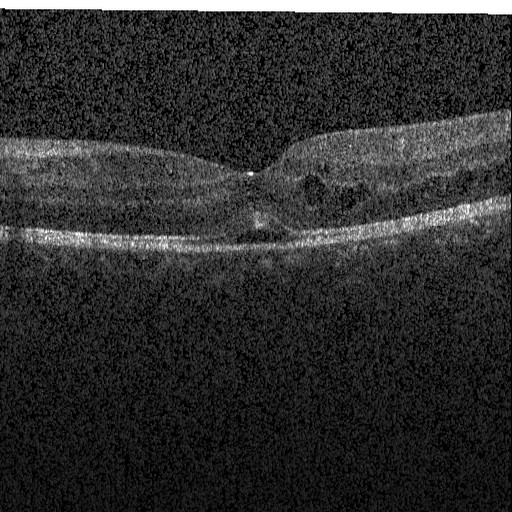

Impression: DME.